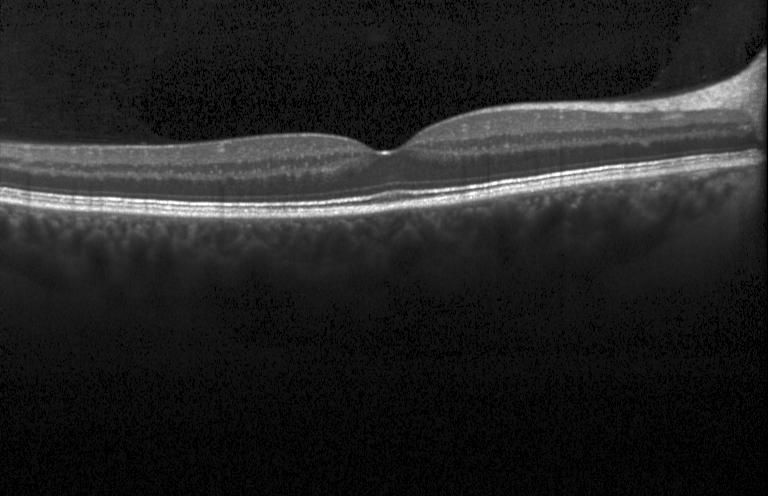
Macular OCT demonstrating no CNV, DME, or drusen.